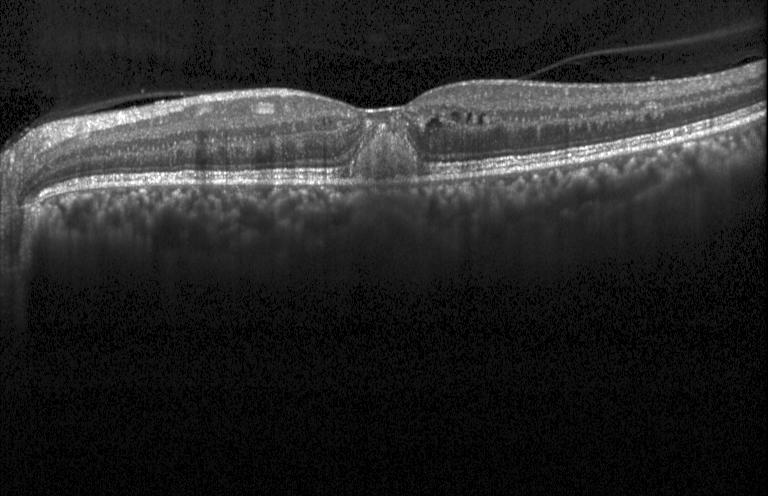 Through the macula. Optical coherence tomography B-scan. SD-OCT
Finding: CNV.